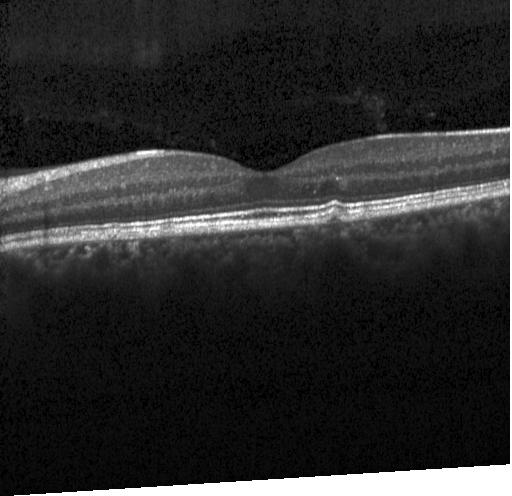 Optical coherence tomography B-scan, macular scan
Dx: sub-RPE drusenoid deposits.